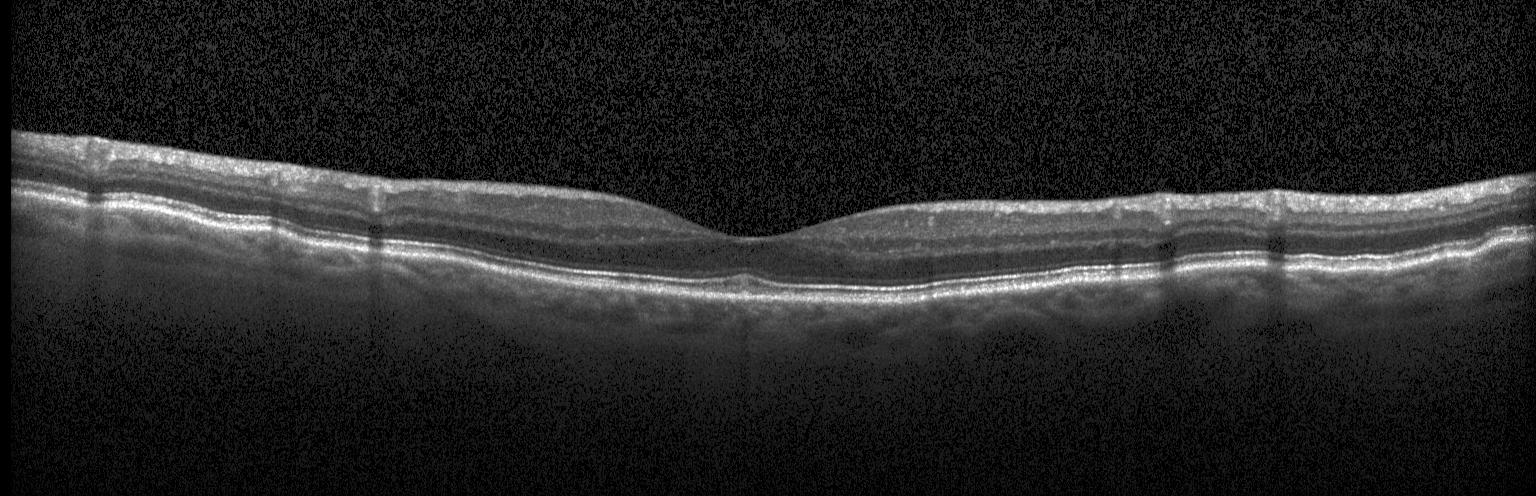 OCT scan showing no evidence of choroidal neovascularization, diabetic macular edema, or drusen.